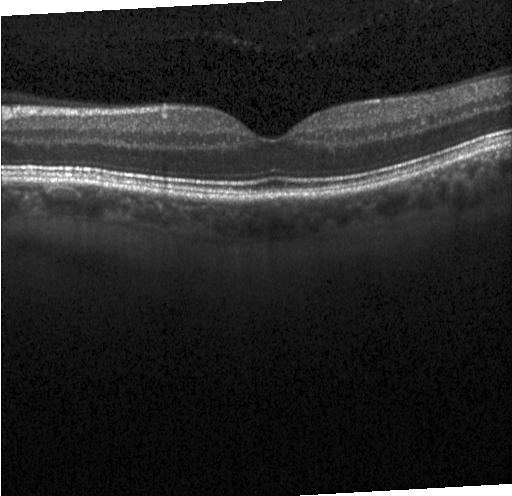 Diagnosis: no choroidal neovascularization, diabetic macular edema, or drusen.